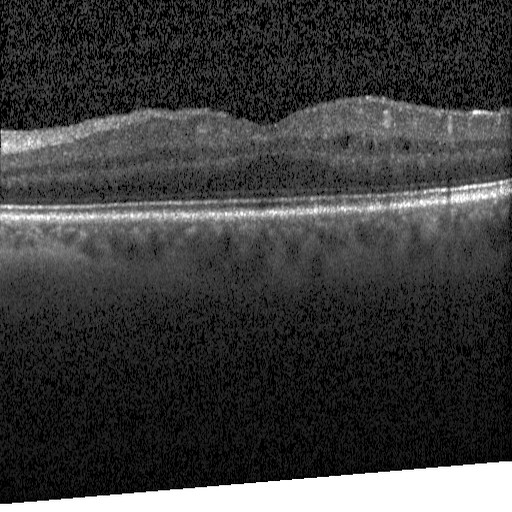

Finding: diabetic macular edema (DME).